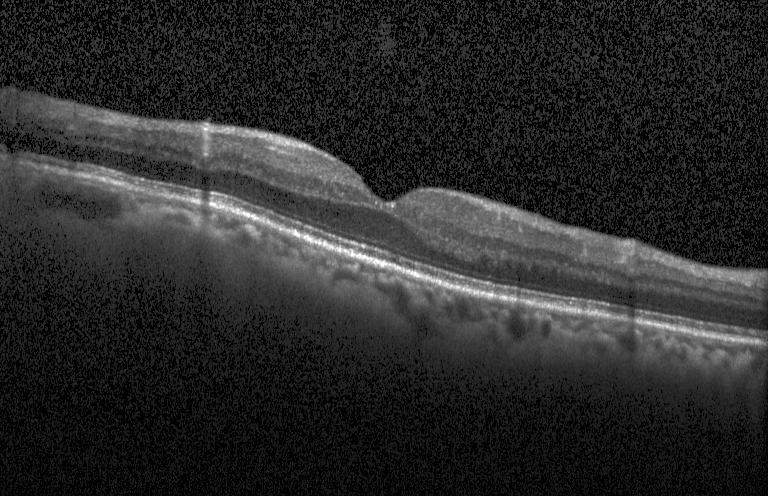 Through the macula; OCT line scan. Impression: no CNV, DME, or drusen.